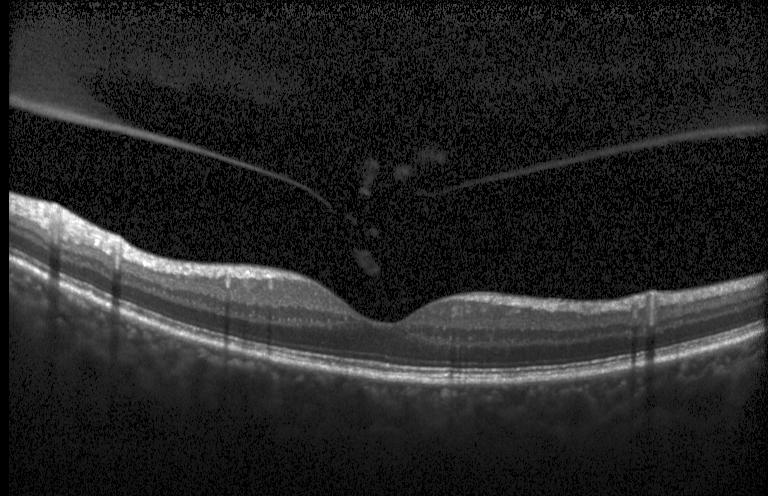

OCT B-scan, Heidelberg Spectralis OCT system, centered on the fovea, spectral-domain OCT.
Diagnosis: neither choroidal neovascularization, diabetic macular edema, nor drusen.